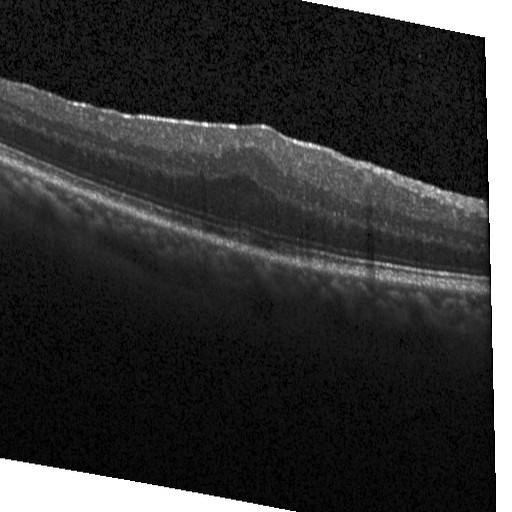

Impression: diabetic macular edema.